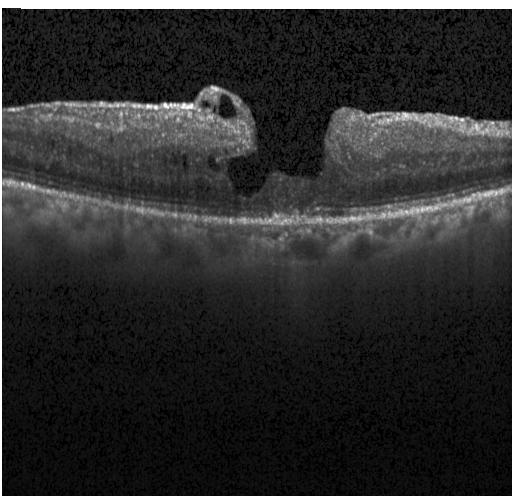

Macular scan · SD-OCT · Heidelberg Spectralis · retinal OCT cross-section.
Diagnosis: DME.